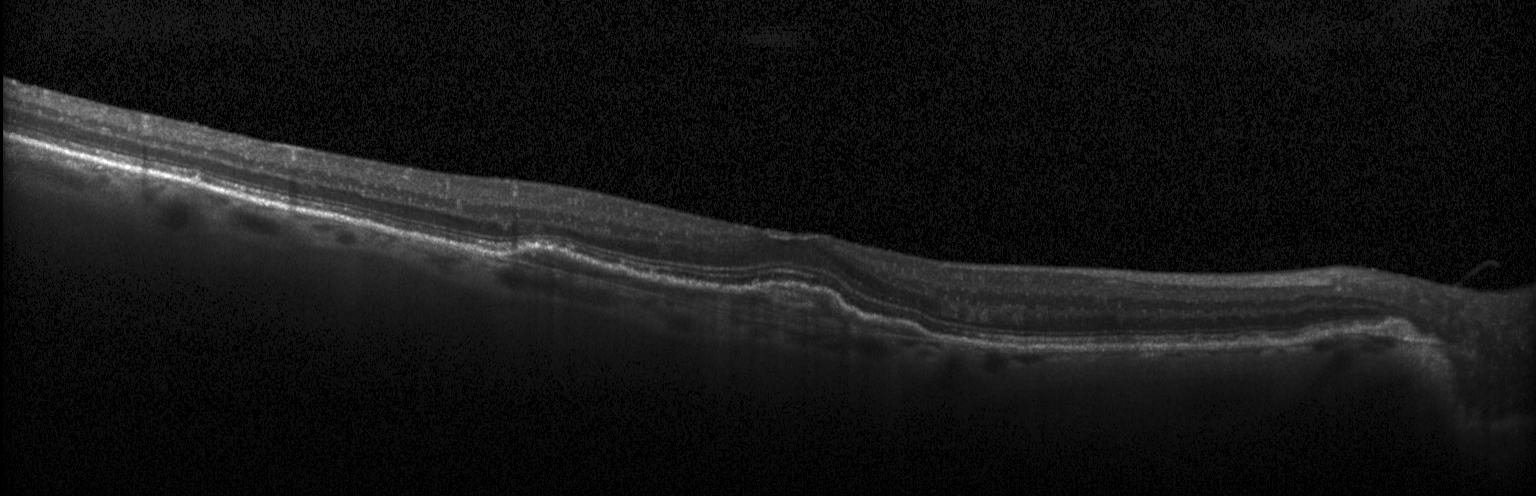 Fovea-centered; OCT line scan; SD-OCT — Impression: choroidal neovascularization.